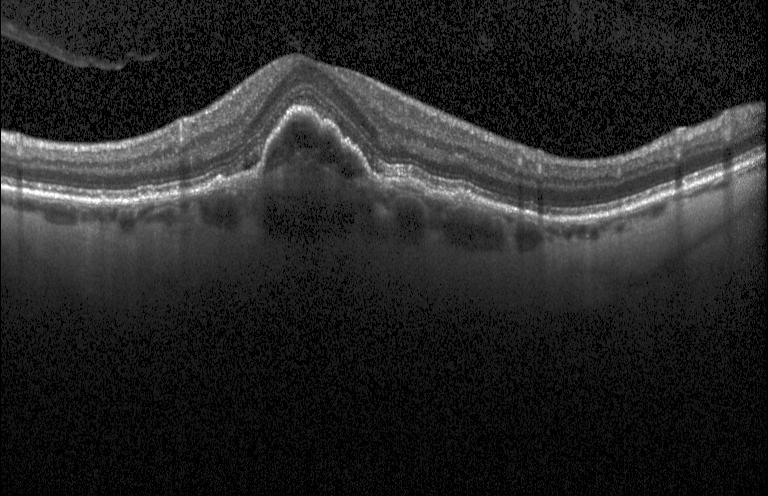
Impression: choroidal neovascularization.